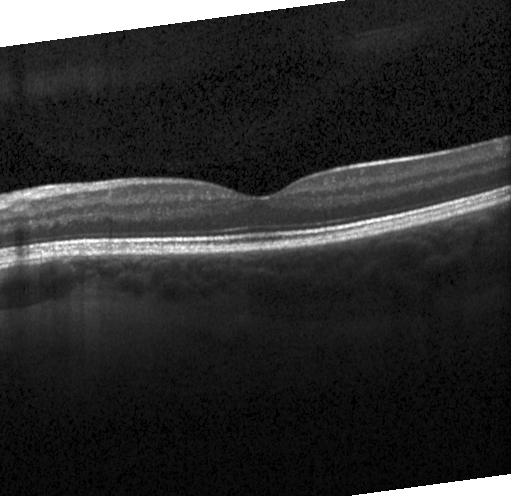

Dx: no evidence of choroidal neovascularization, diabetic macular edema, or drusen.